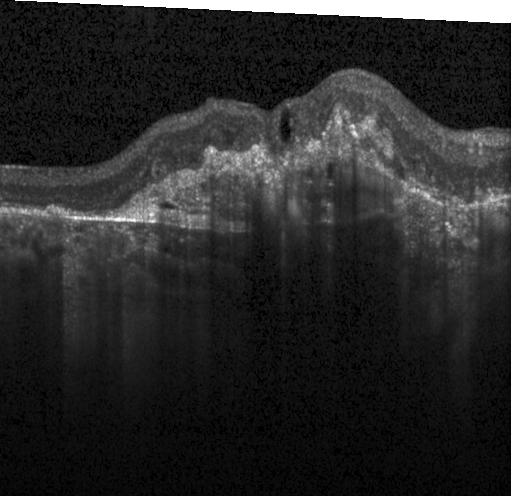 Centered on the fovea; spectral-domain OCT; Heidelberg Spectralis OCT system; retinal OCT B-scan. This B-scan demonstrates a choroidal neovascular membrane.